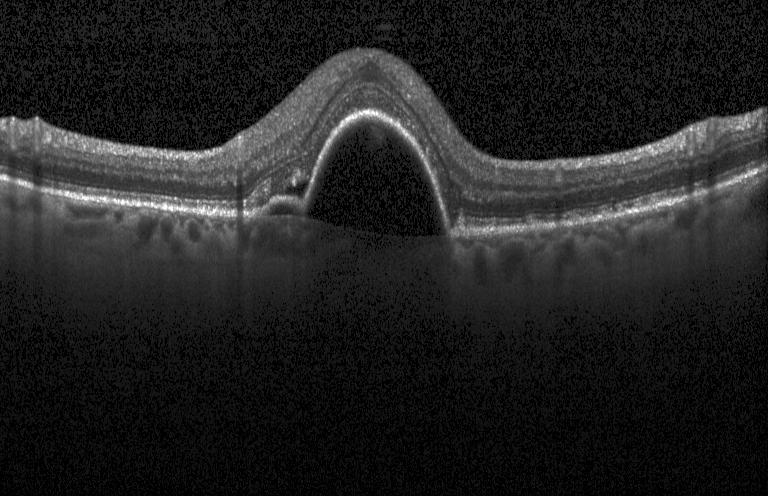

OCT finding: choroidal neovascularization (CNV).